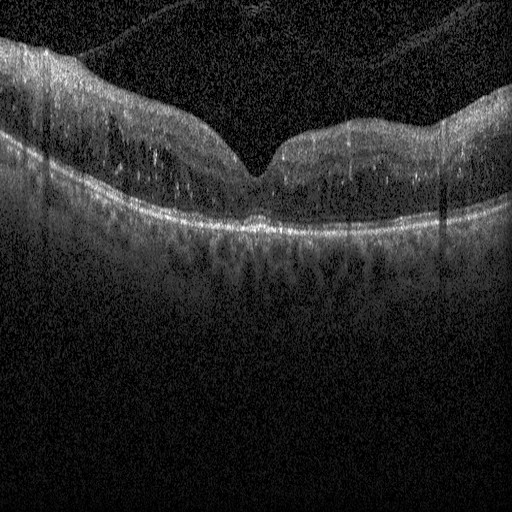
Fovea-centered. Spectral-domain OCT. Heidelberg Spectralis OCT system. OCT B-scan
Finding: DME.